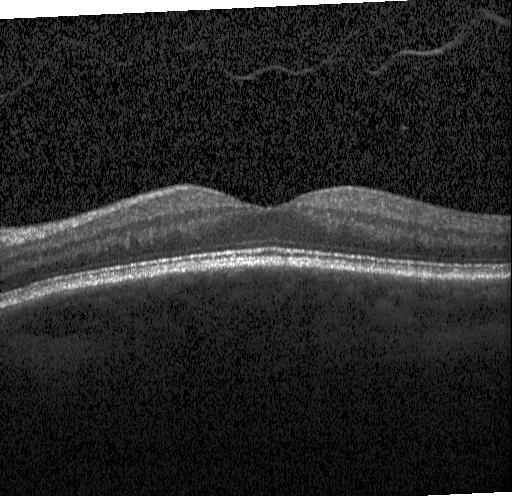
Heidelberg Spectralis, OCT B-scan
Impression: neither choroidal neovascularization, diabetic macular edema, nor drusen.